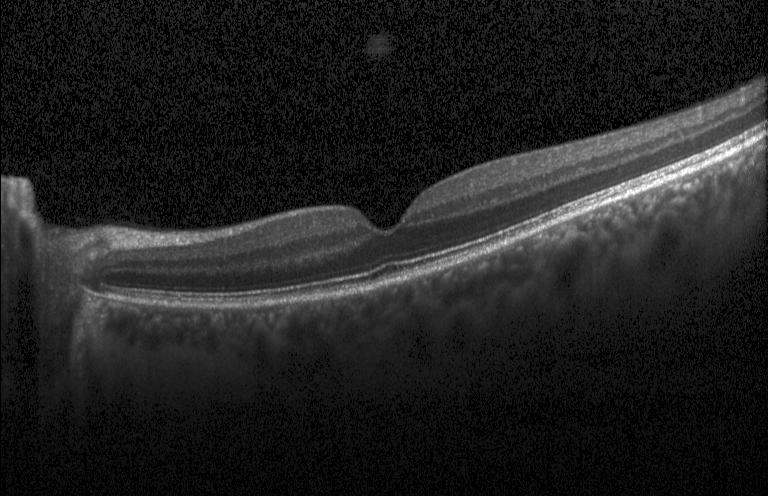
Retinal OCT B-scan · Heidelberg Spectralis OCT system. Diagnosis: no CNV, no DME, and no drusen.